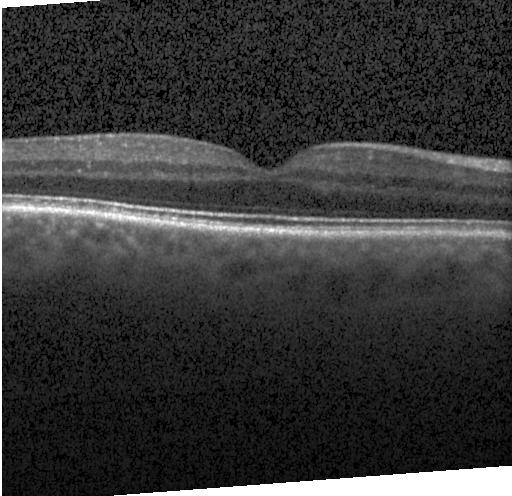

Horizontal scan through the fovea. OCT line scan. Spectral-domain optical coherence tomography. Instrument: Heidelberg Spectralis.
Dx: no evidence of choroidal neovascularization, diabetic macular edema, or drusen.